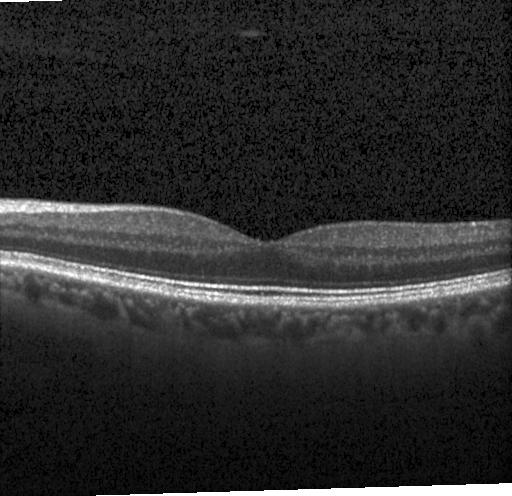
Finding: no CNV, no DME, and no drusen.